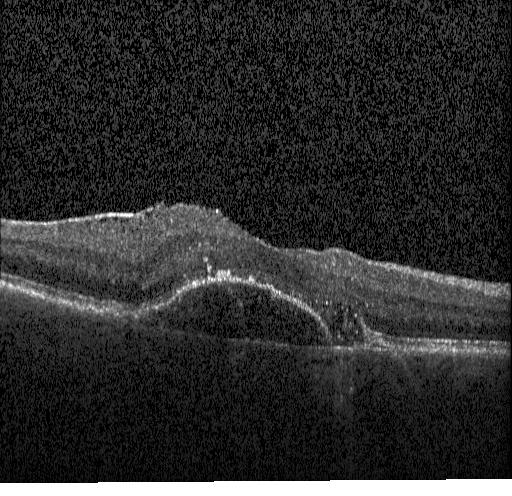
Spectral-domain OCT B-scan: choroidal neovascularization.